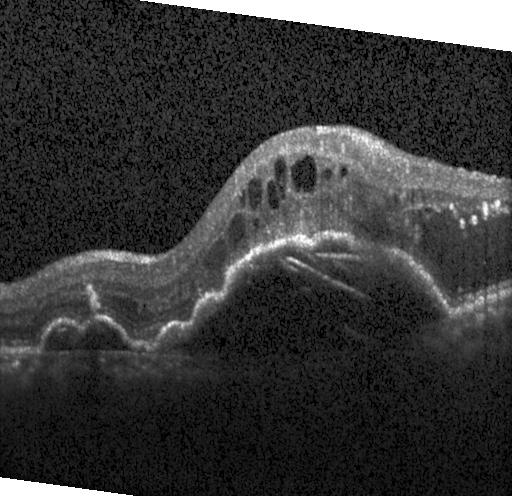 Instrument: Heidelberg Spectralis, horizontal scan through the fovea, optical coherence tomography scan.
Dx: choroidal neovascularization (CNV).